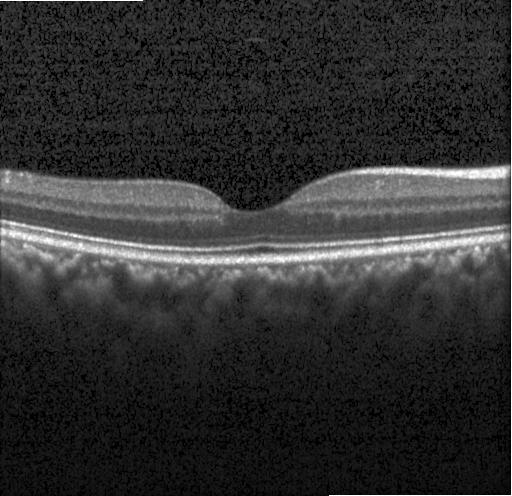

This B-scan demonstrates neither choroidal neovascularization, diabetic macular edema, nor drusen.